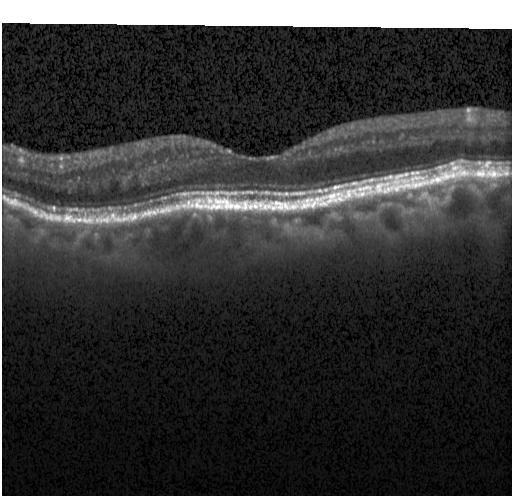 Macular OCT: no choroidal neovascularization, no diabetic macular edema, and no drusen.